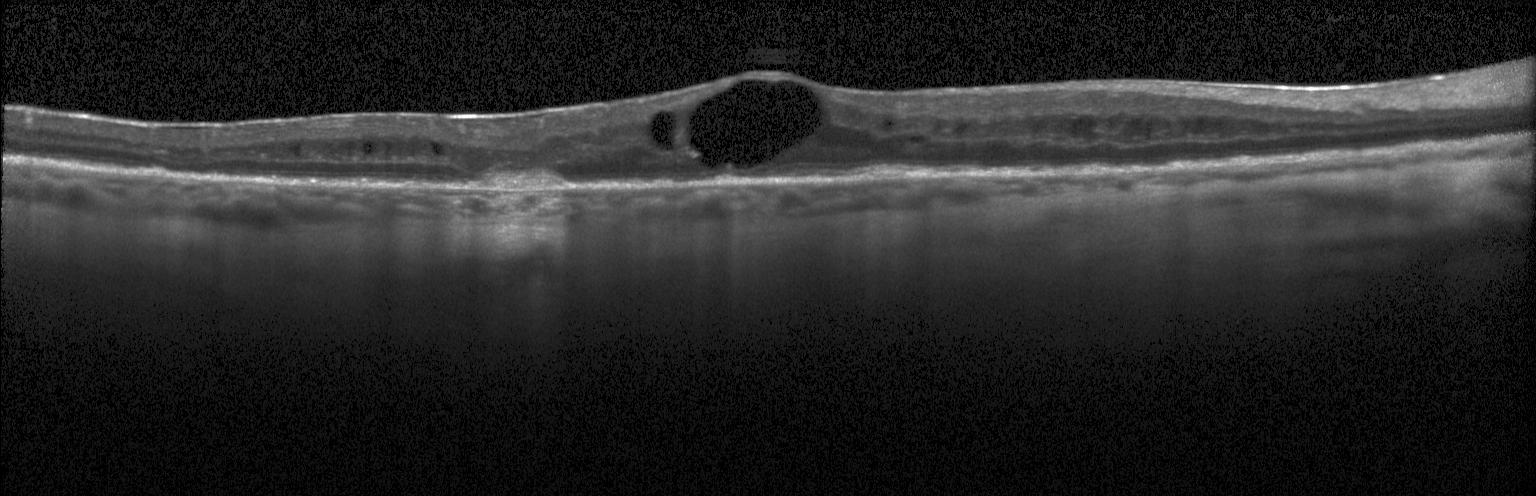 Retinal OCT cross-section; SD-OCT
The scan shows a choroidal neovascular membrane.